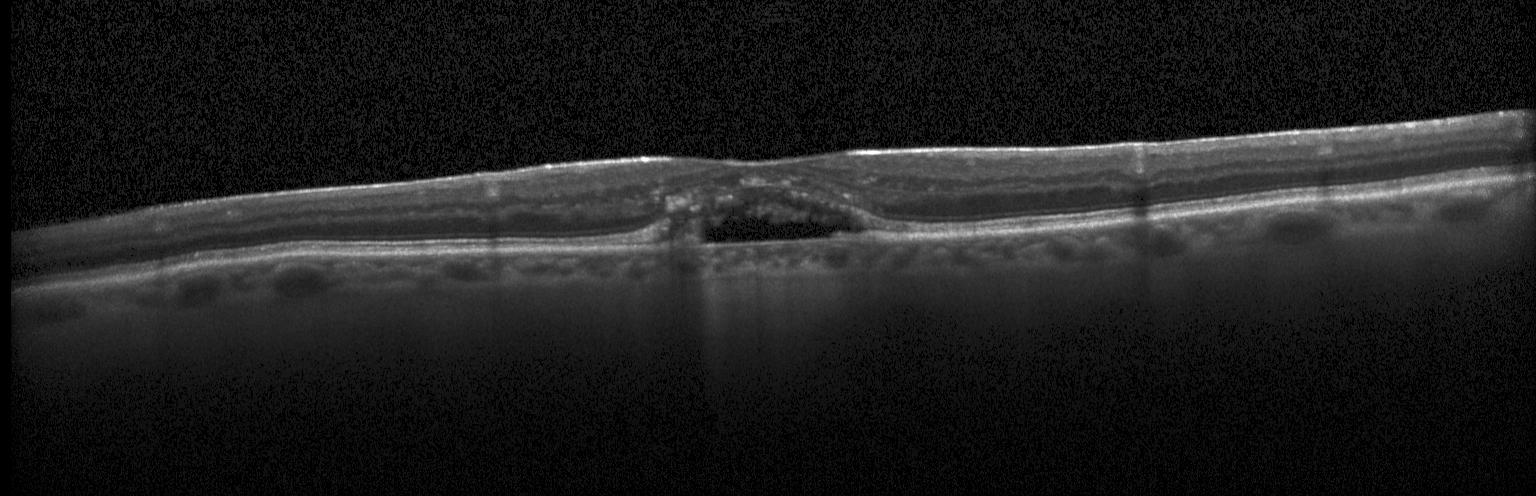 Dx: a choroidal neovascular membrane.